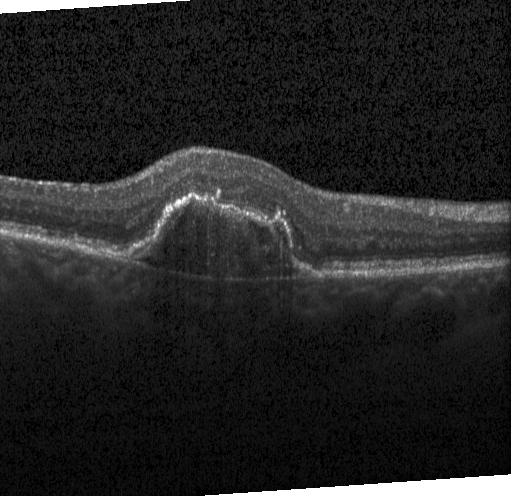
Retinal OCT cross-section. A choroidal neovascular membrane.